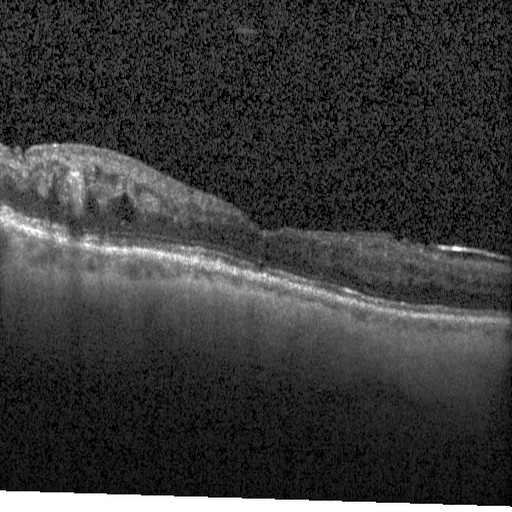 Optical coherence tomography scan; spectral-domain optical coherence tomography; fovea-centered — The scan shows diabetic macular edema (DME).